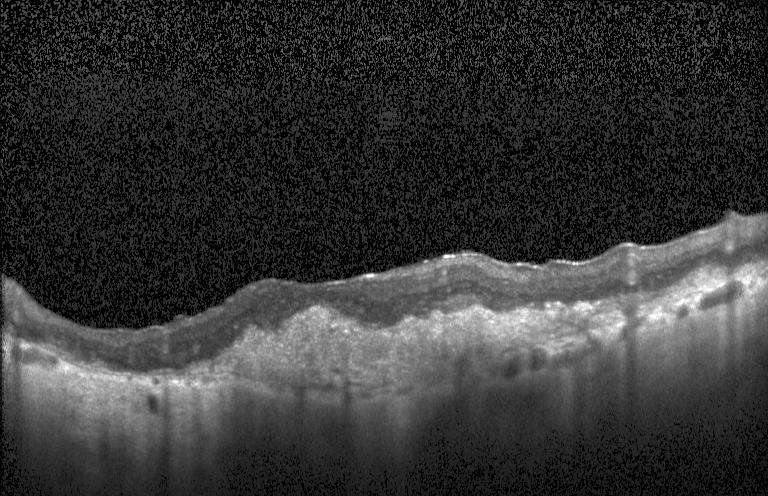 Retinal OCT B-scan. Diagnosis: choroidal neovascularization (CNV).